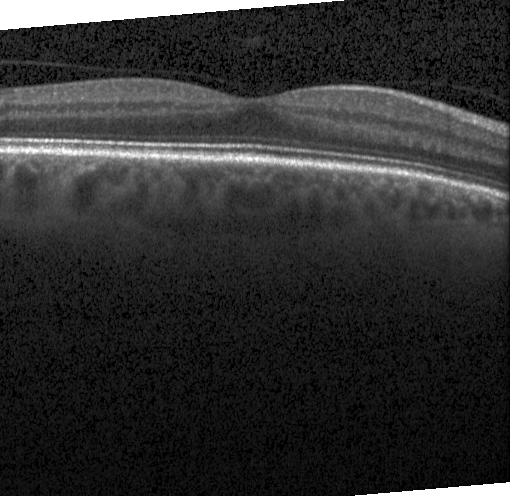

Optical coherence tomography scan, Heidelberg Spectralis OCT system, spectral-domain OCT. Diagnosis: no choroidal neovascularization, diabetic macular edema, or drusen.